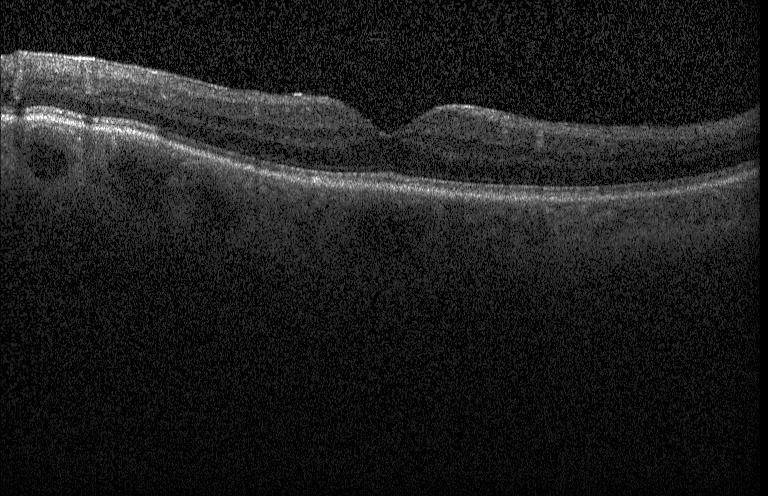
OCT scan showing neither CNV, DME, nor drusen.